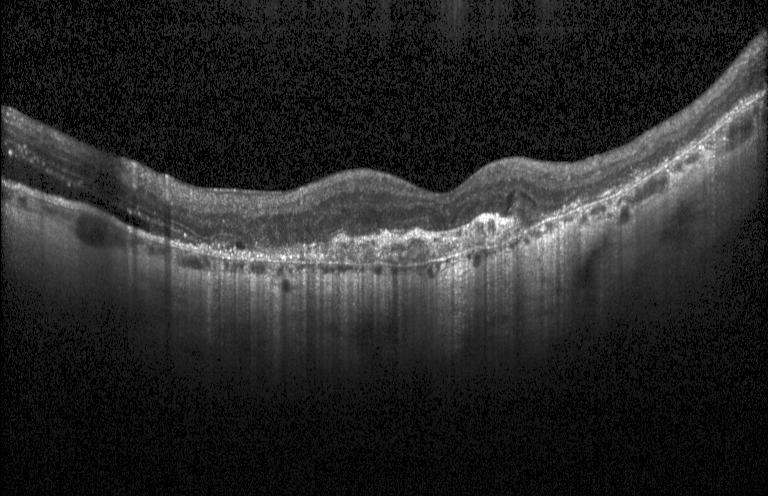 Optical coherence tomography scan. This B-scan demonstrates a choroidal neovascular membrane.